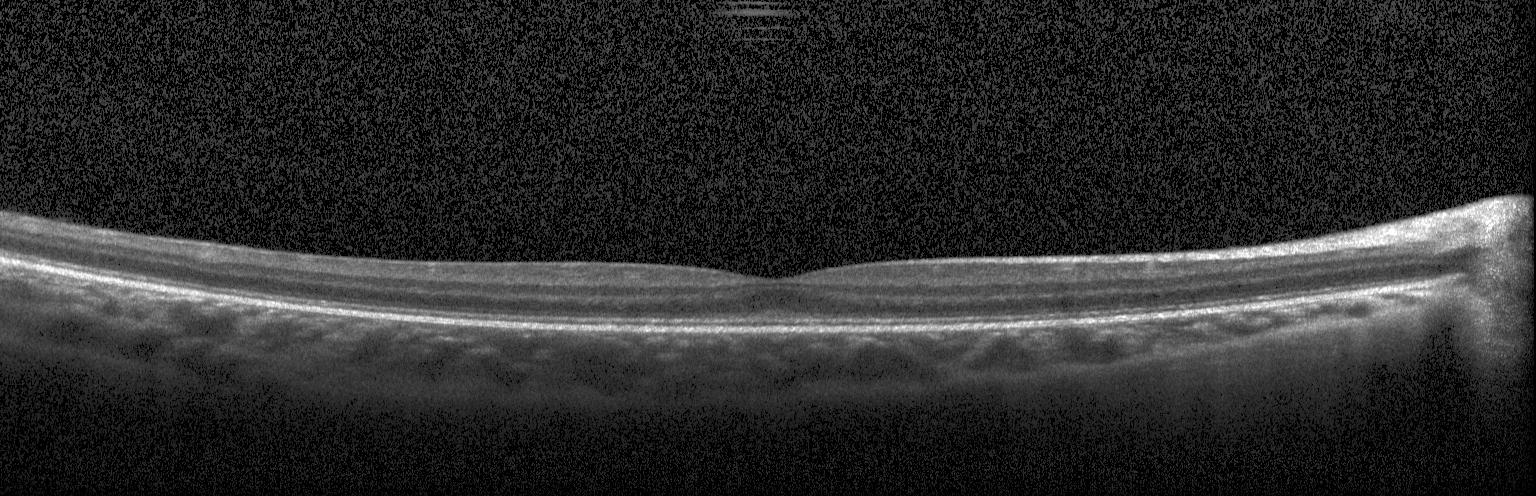 SD-OCT, retinal OCT B-scan, through the macula — Finding: no CNV, DME, or drusen.